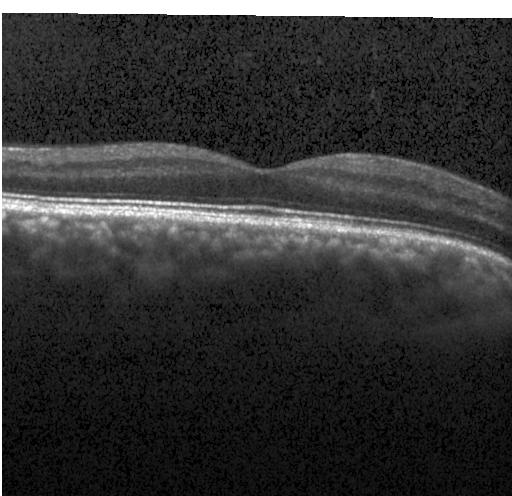
Retinal OCT cross-section; Heidelberg Spectralis; fovea-centered; spectral-domain optical coherence tomography
OCT finding: neither choroidal neovascularization, diabetic macular edema, nor drusen.